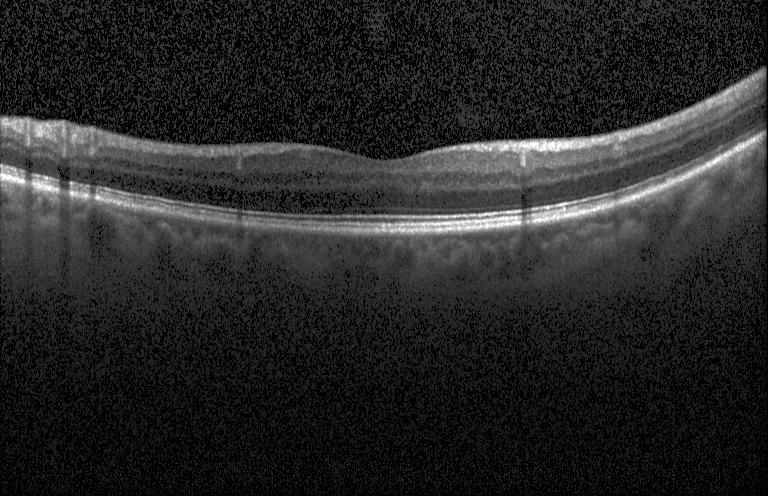 OCT line scan. Dx: no choroidal neovascularization, no diabetic macular edema, and no drusen.